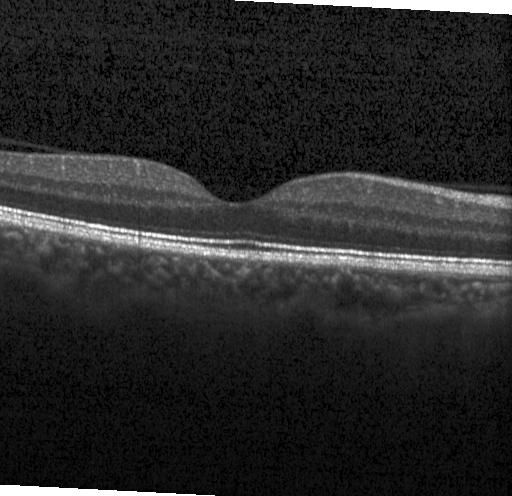
Finding: no evidence of CNV, DME, or drusen.